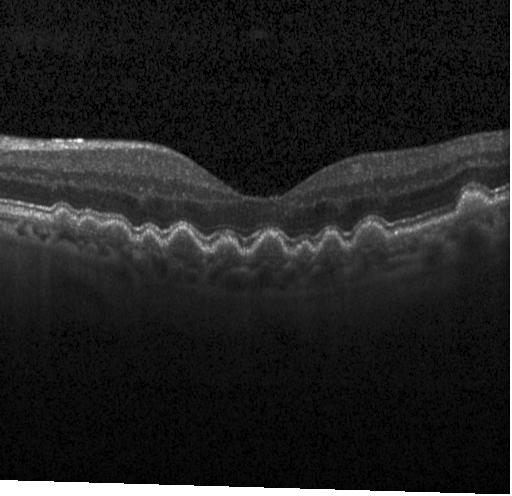 Optical coherence tomography scan · spectral-domain OCT — Assessment: drusen.